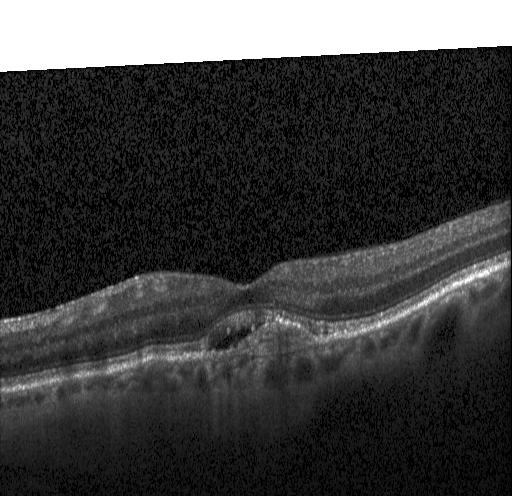
Diagnosis: a choroidal neovascular membrane.